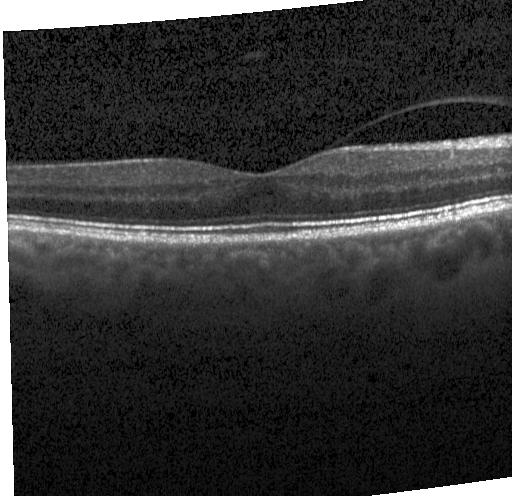 Retinal OCT cross-section · spectral-domain OCT.
OCT finding: neither choroidal neovascularization, diabetic macular edema, nor drusen.